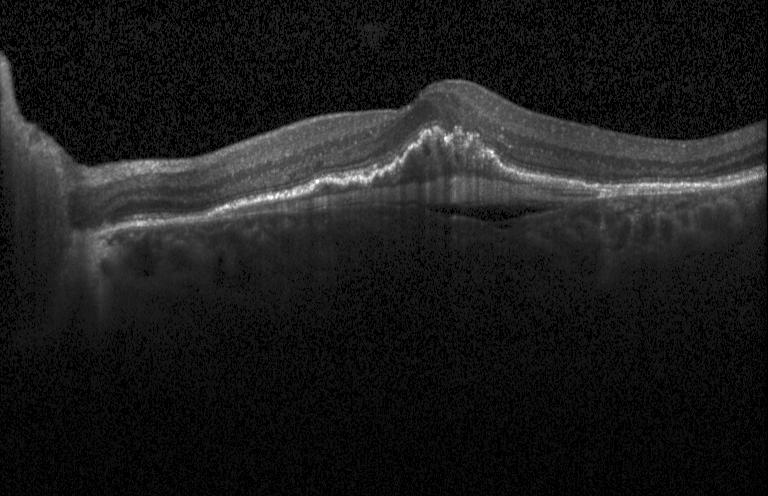 Heidelberg Spectralis · SD-OCT · optical coherence tomography scan.
Assessment: a choroidal neovascular membrane.